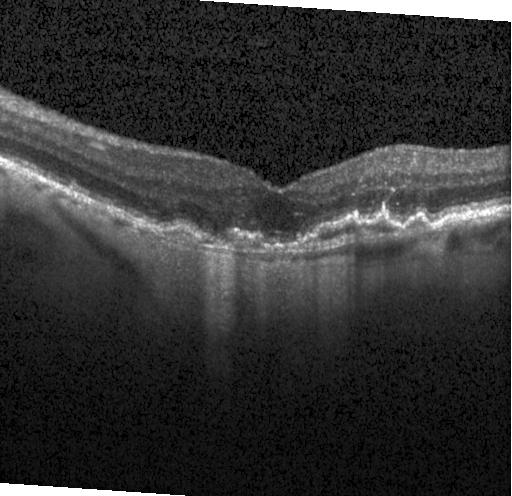

Macular OCT demonstrating choroidal neovascularization.